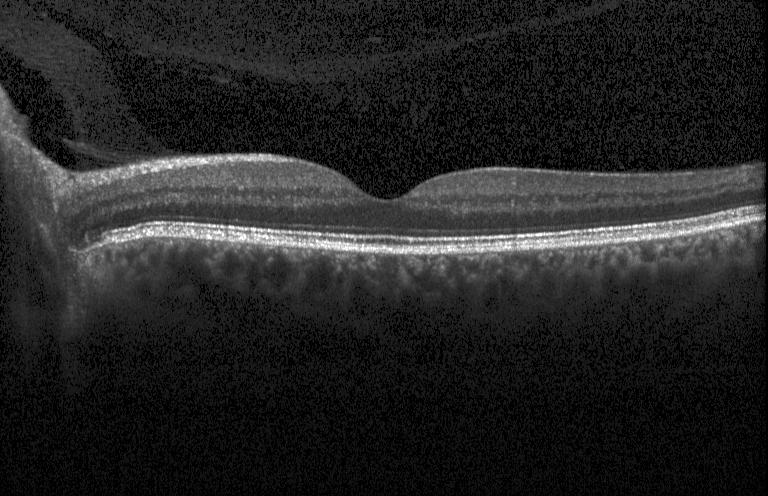 This B-scan demonstrates no choroidal neovascularization, diabetic macular edema, or drusen.